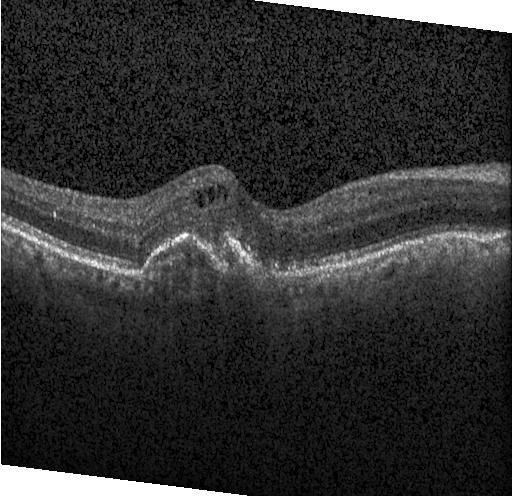
Optical coherence tomography scan, spectral-domain OCT. OCT finding: a choroidal neovascular membrane.